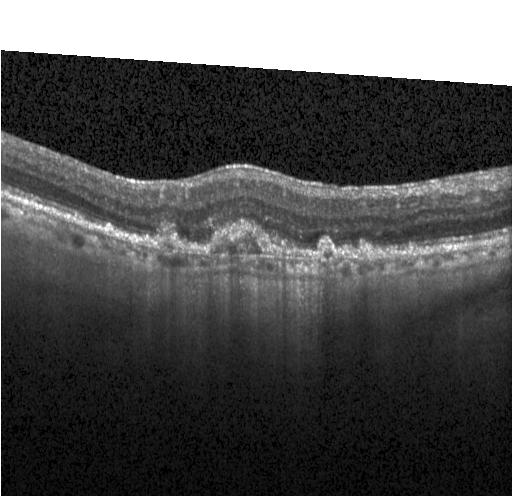

Retinal OCT cross-section; centered on the fovea; spectral-domain optical coherence tomography
Diagnosis: a choroidal neovascular membrane.